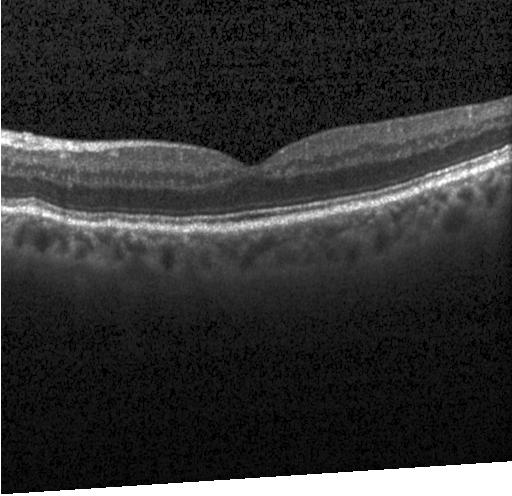 Optical coherence tomography B-scan. Spectral-domain OCT — Finding: neither choroidal neovascularization, diabetic macular edema, nor drusen.